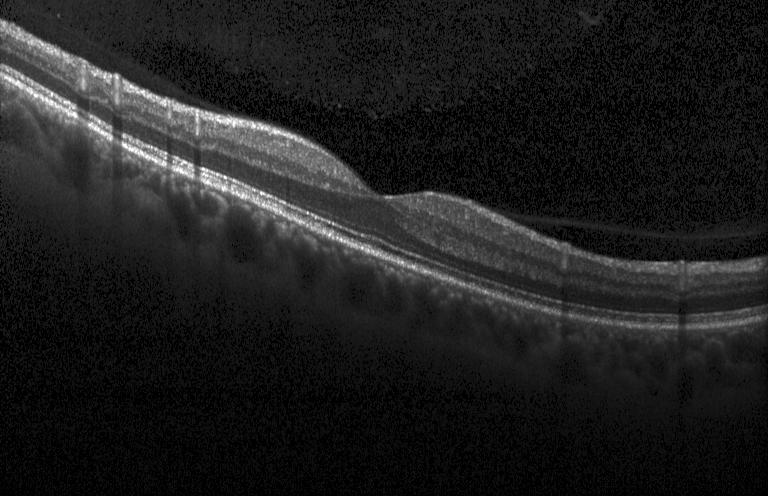

Spectral-domain OCT · OCT line scan — Finding: no choroidal neovascularization, no diabetic macular edema, and no drusen.